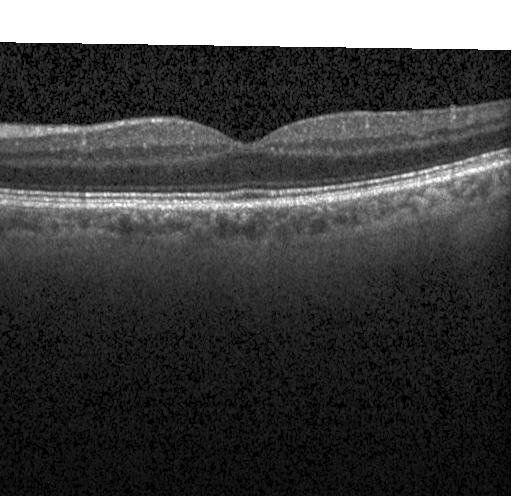

SD-OCT, OCT line scan. Impression: no choroidal neovascularization, no diabetic macular edema, and no drusen.